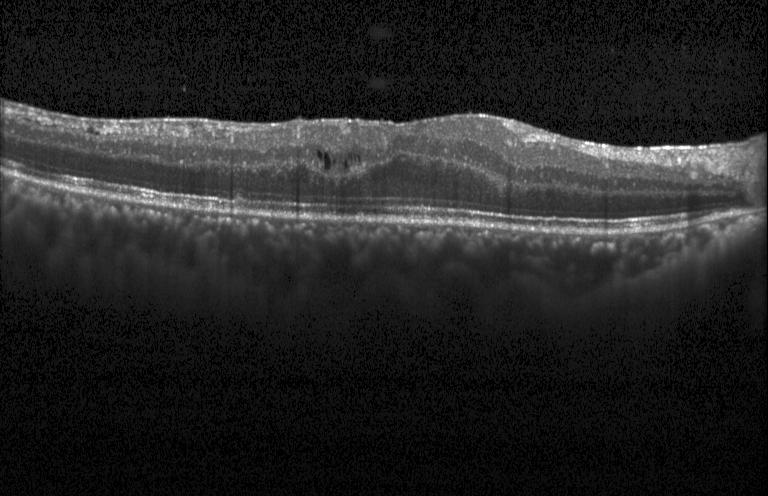
Instrument: Heidelberg Spectralis · horizontal scan through the fovea · OCT line scan — The scan shows DME.